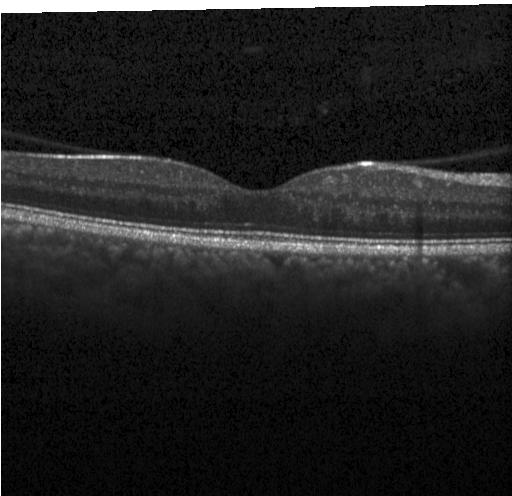
Acquired on a Heidelberg Spectralis. Spectral-domain optical coherence tomography. Optical coherence tomography B-scan. Horizontal scan through the fovea. Diagnosis: no choroidal neovascularization, diabetic macular edema, or drusen.